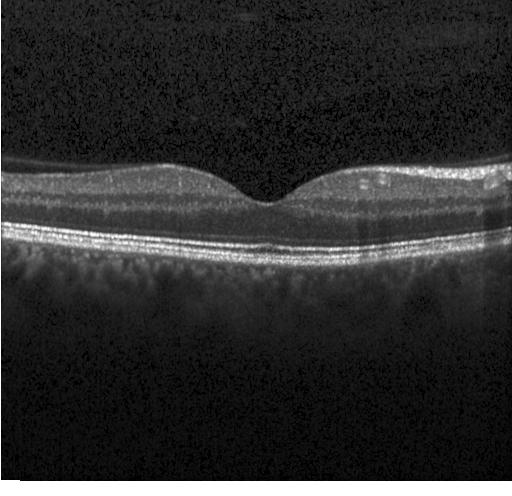
Finding: no evidence of choroidal neovascularization, diabetic macular edema, or drusen.